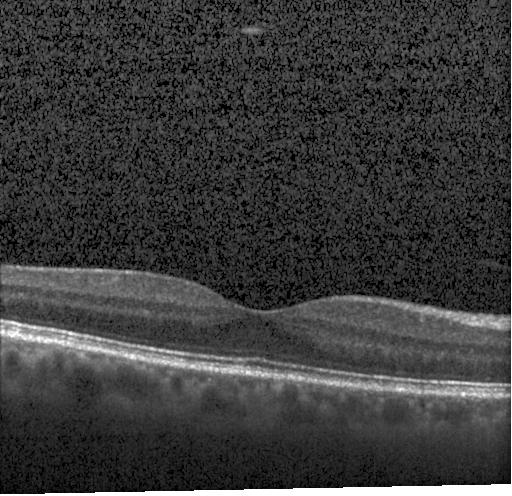
Finding: no choroidal neovascularization, diabetic macular edema, or drusen.